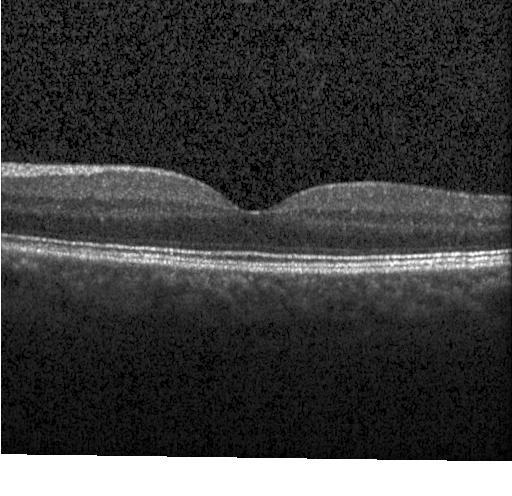

OCT line scan. Impression: neither choroidal neovascularization, diabetic macular edema, nor drusen.